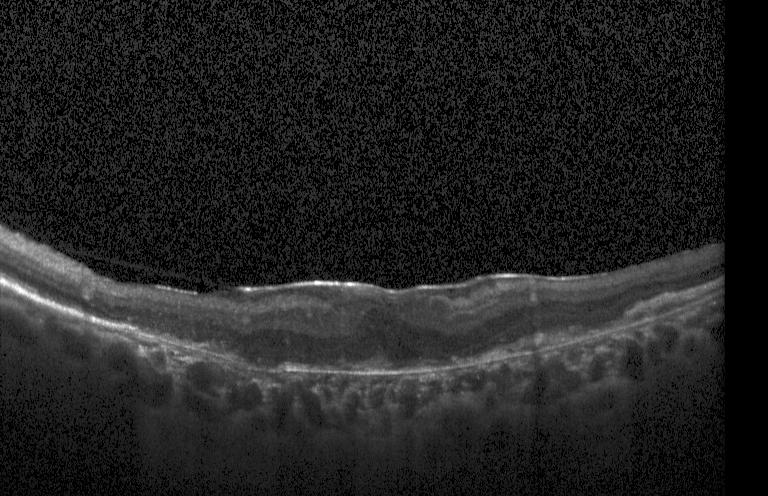
Dx: choroidal neovascularization (CNV).